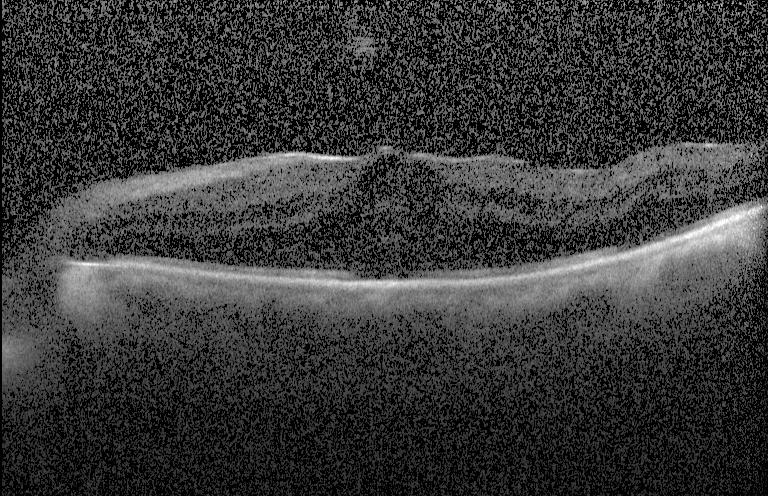 Retinal OCT B-scan.
This B-scan demonstrates DME.